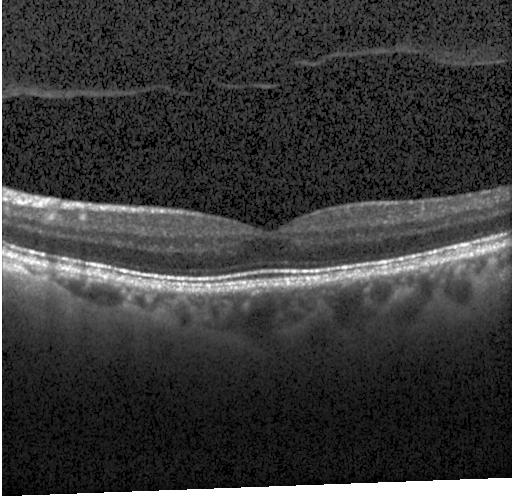
Spectral-domain OCT. Retinal OCT B-scan. Fovea-centered. Acquired on a Heidelberg Spectralis.
Dx: no choroidal neovascularization, no diabetic macular edema, and no drusen.